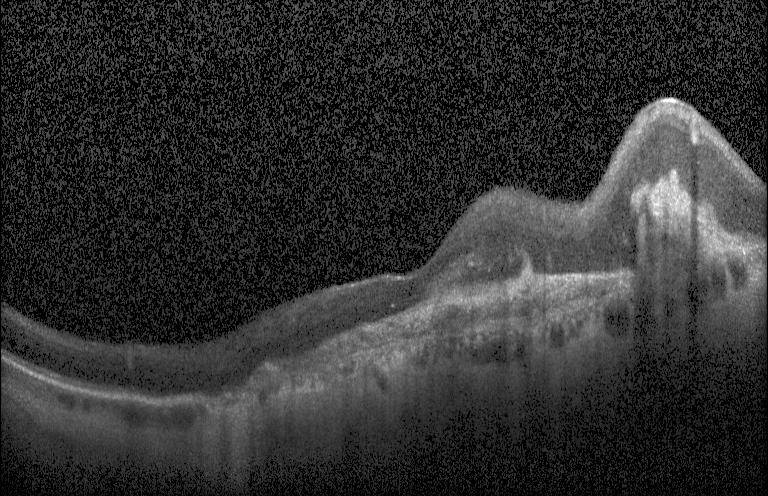
Retinal OCT B-scan · spectral-domain optical coherence tomography. This B-scan demonstrates a choroidal neovascular membrane.